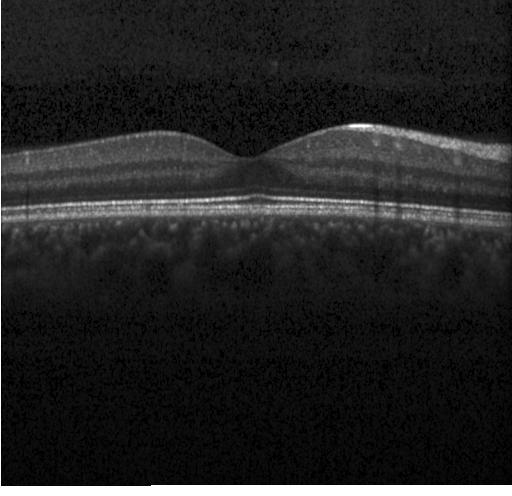

OCT line scan. Heidelberg Spectralis — Finding: no choroidal neovascularization, diabetic macular edema, or drusen.